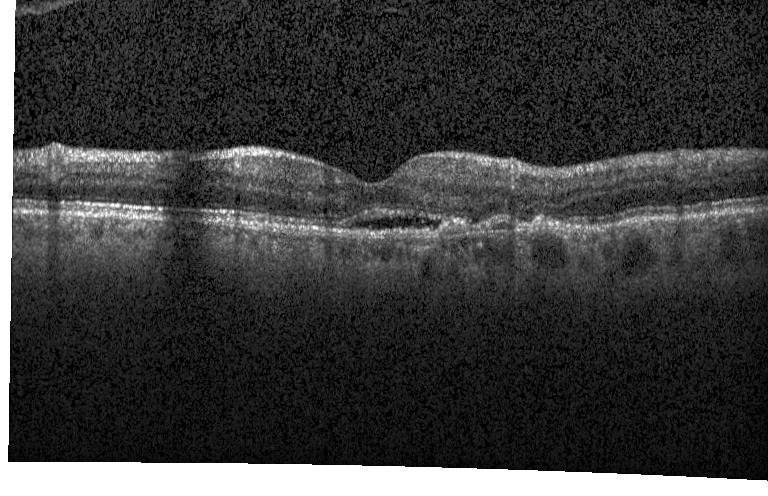
Retinal OCT cross-section.
This B-scan demonstrates choroidal neovascularization.